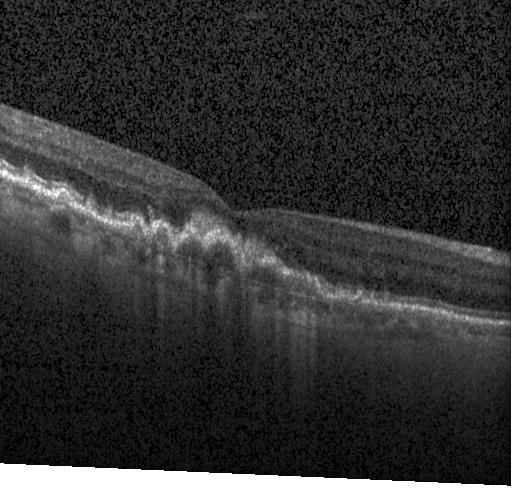

Impression: a choroidal neovascular membrane.